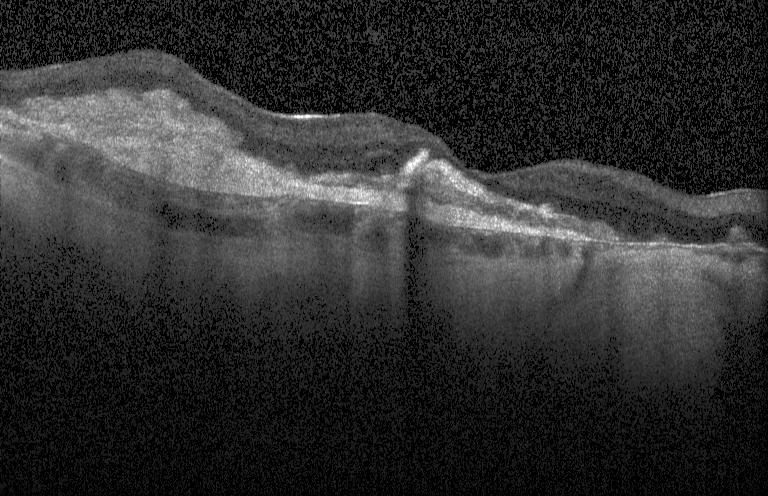 OCT finding: CNV.